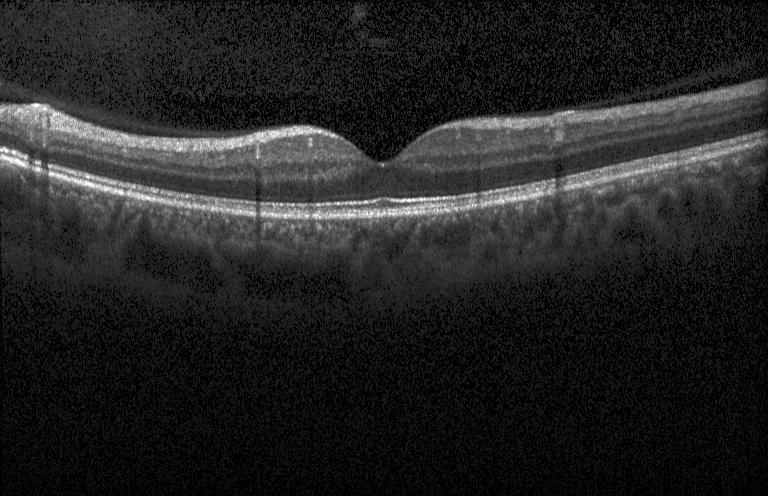
Retinal OCT B-scan
Finding: no choroidal neovascularization, no diabetic macular edema, and no drusen.